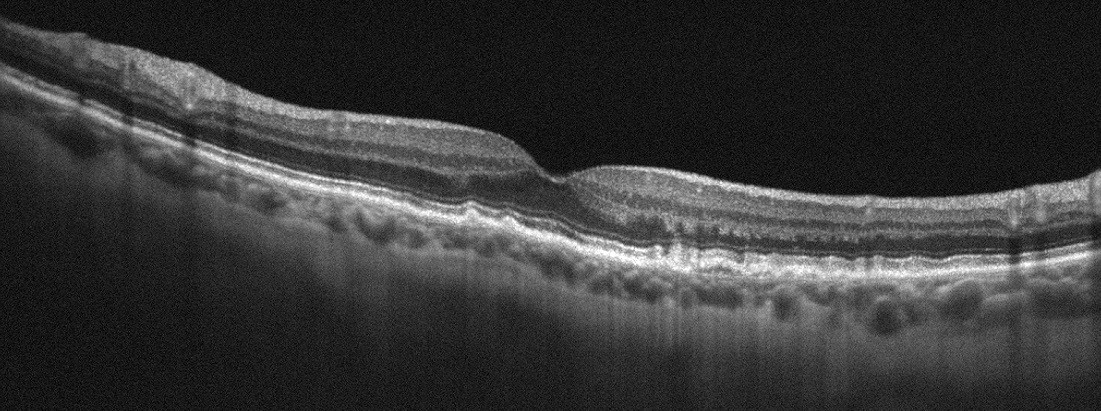 Through the macula. Instrument: Optovue Avanti RTVue XR. Retinal OCT cross-section
OCT finding: age-related macular degeneration.